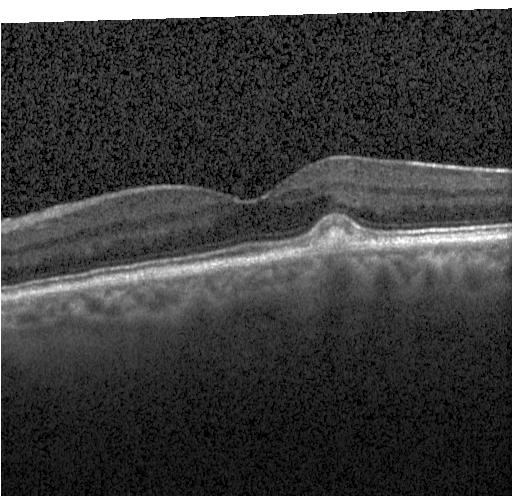 Diagnosis: sub-RPE drusenoid deposits.